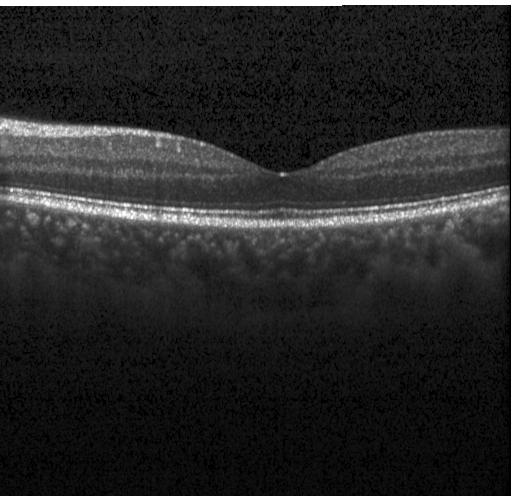

Macular OCT demonstrating neither CNV, DME, nor drusen.